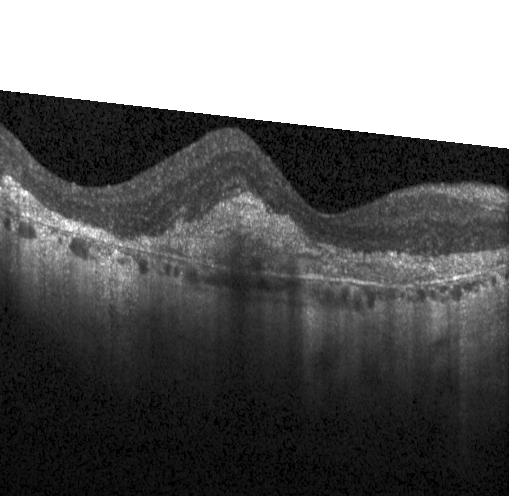
Optical coherence tomography B-scan
The scan shows a choroidal neovascular membrane.